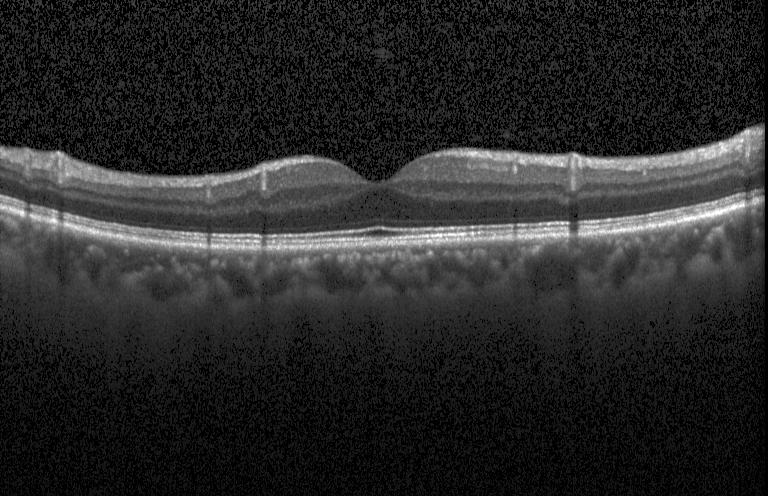

Optical coherence tomography scan, macular scan.
No evidence of CNV, DME, or drusen.